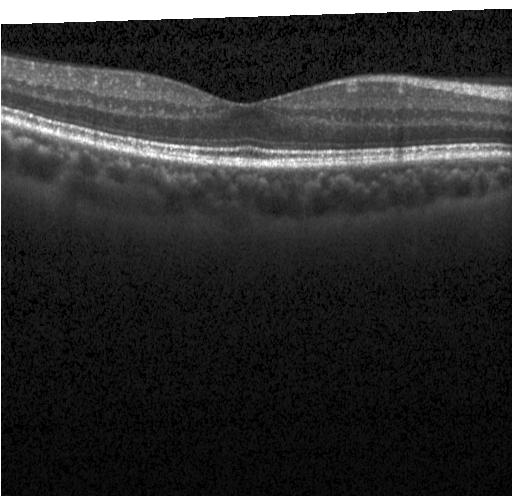 Dx: no choroidal neovascularization, no diabetic macular edema, and no drusen.